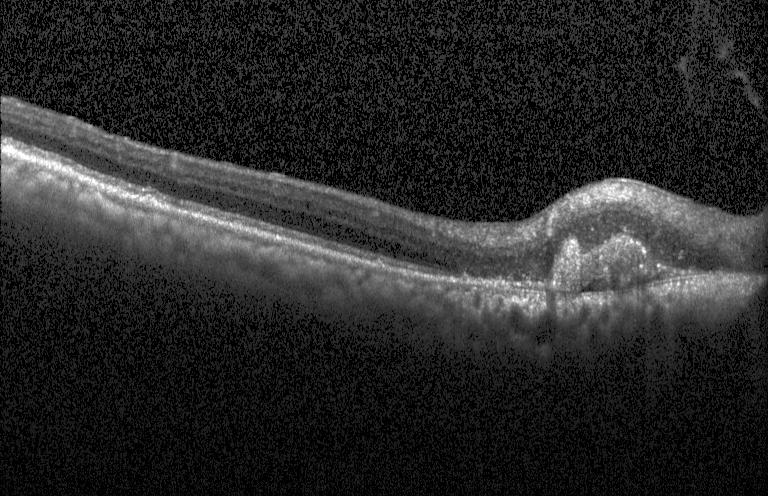

Diagnosis: choroidal neovascularization.